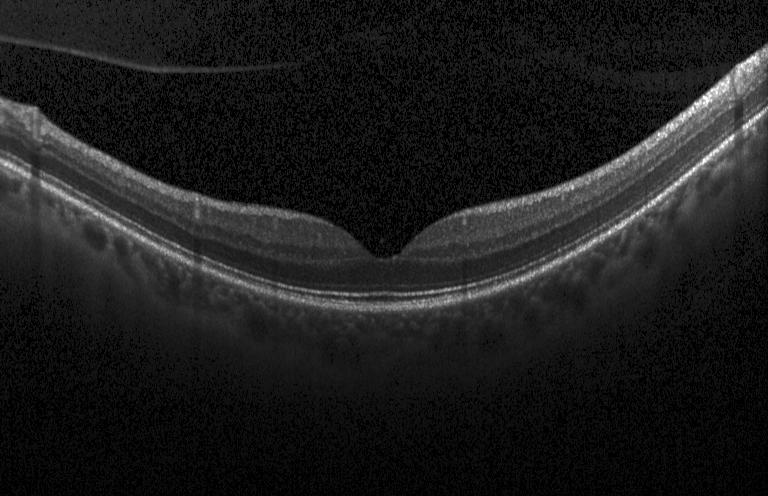
No evidence of choroidal neovascularization, diabetic macular edema, or drusen.